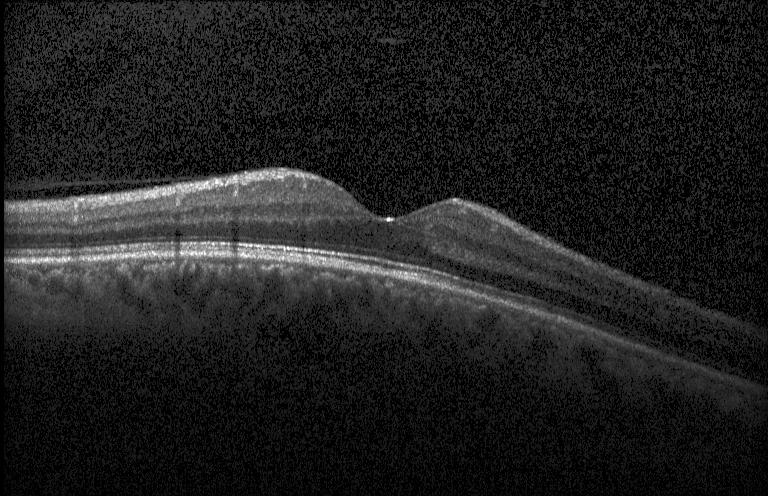

No choroidal neovascularization, no diabetic macular edema, and no drusen.